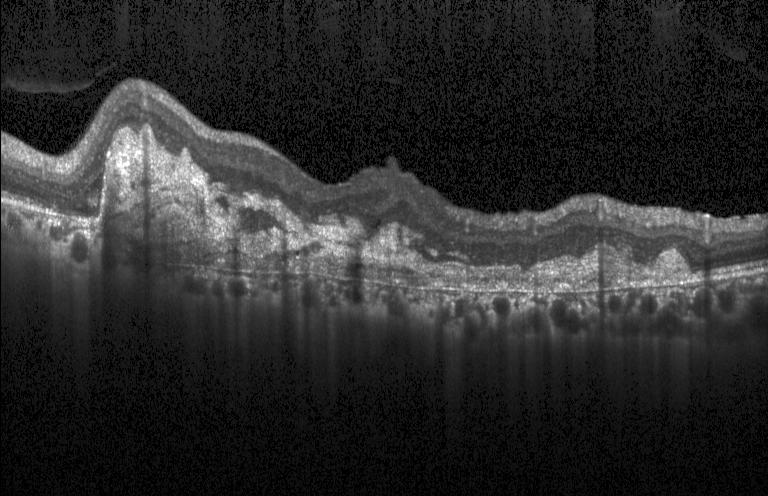
Choroidal neovascularization.